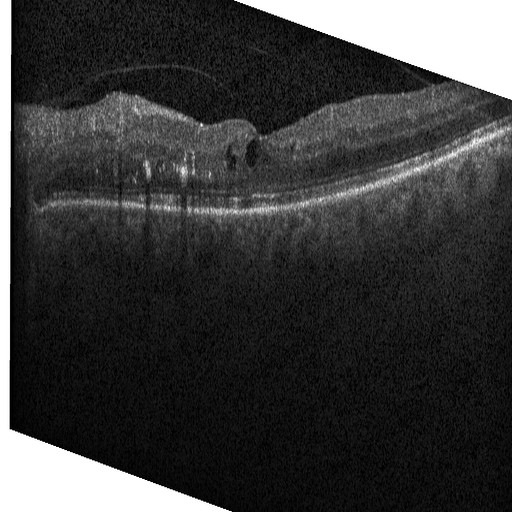

Diagnosis: DME.